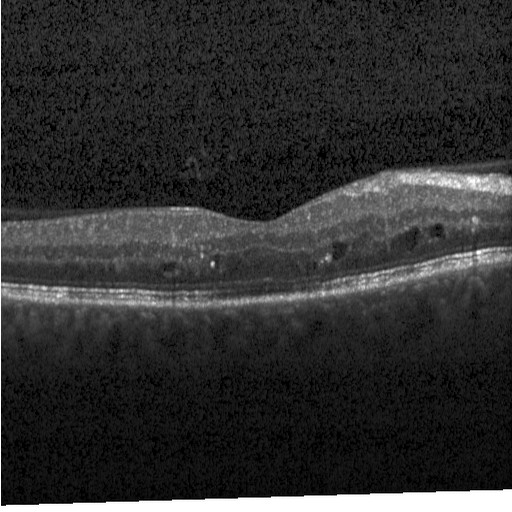 OCT B-scan showing diabetic macular edema (DME).